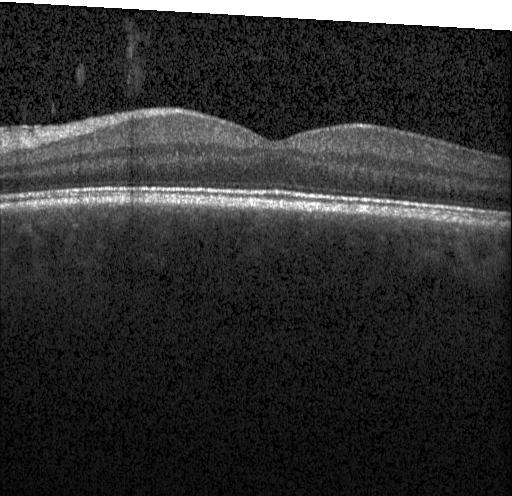
Centered on the fovea, OCT B-scan
Finding: neither choroidal neovascularization, diabetic macular edema, nor drusen.